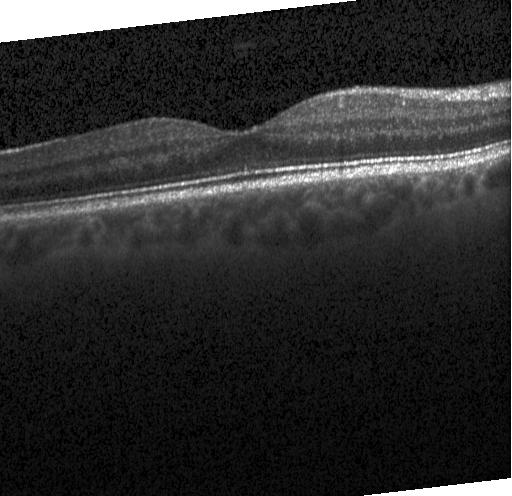
OCT B-scan showing no choroidal neovascularization, no diabetic macular edema, and no drusen.